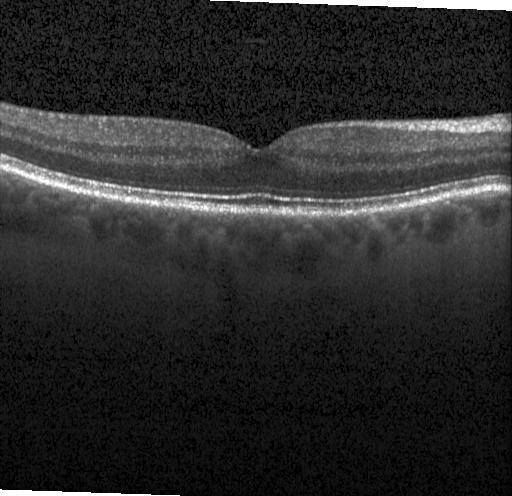

Optical coherence tomography scan, Heidelberg Spectralis OCT system. Finding: neither choroidal neovascularization, diabetic macular edema, nor drusen.